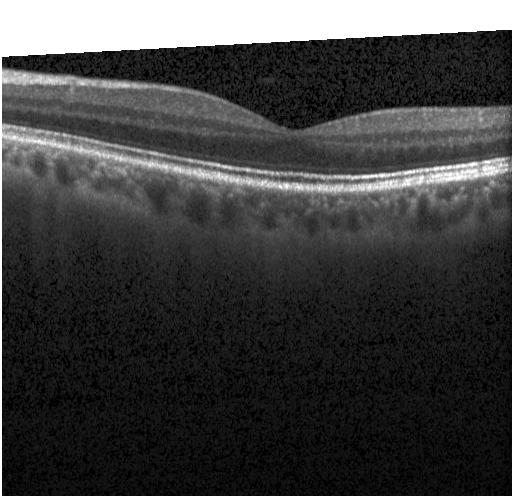

Macular scan. Optical coherence tomography B-scan. Spectral-domain optical coherence tomography. Heidelberg Spectralis
Assessment: no choroidal neovascularization, no diabetic macular edema, and no drusen.